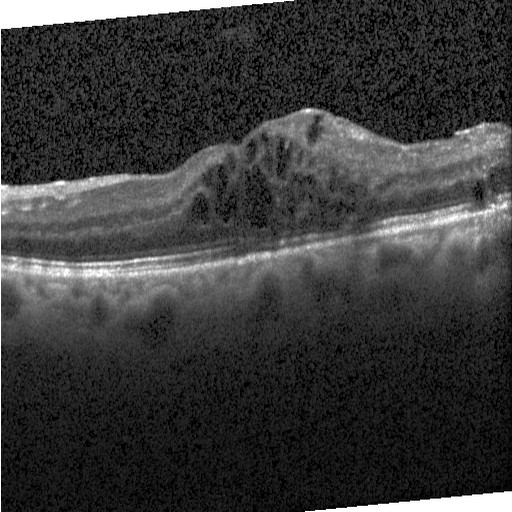
Optical coherence tomography B-scan · macular scan
Impression: diabetic macular edema (DME).